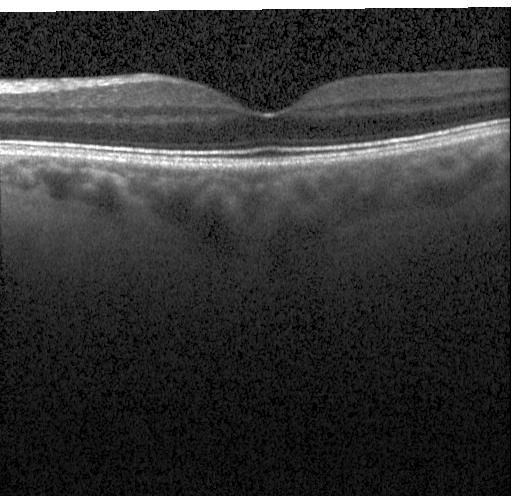
Retinal OCT cross-section, Heidelberg Spectralis, horizontal scan through the fovea. Finding: no choroidal neovascularization, no diabetic macular edema, and no drusen.